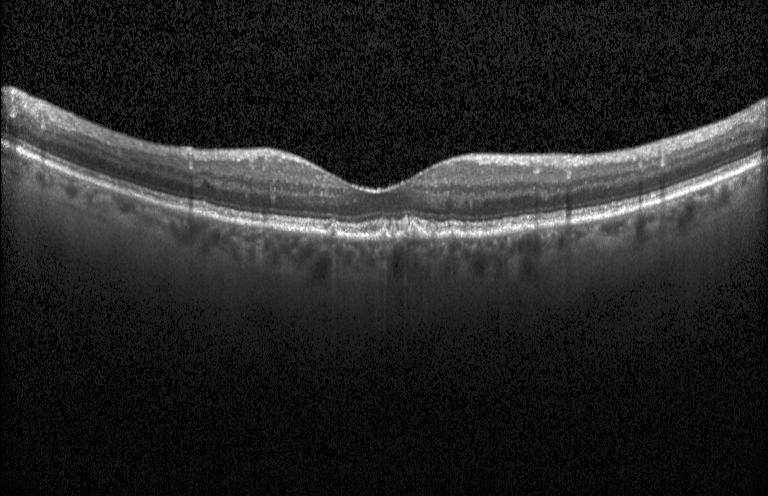
Drusen.